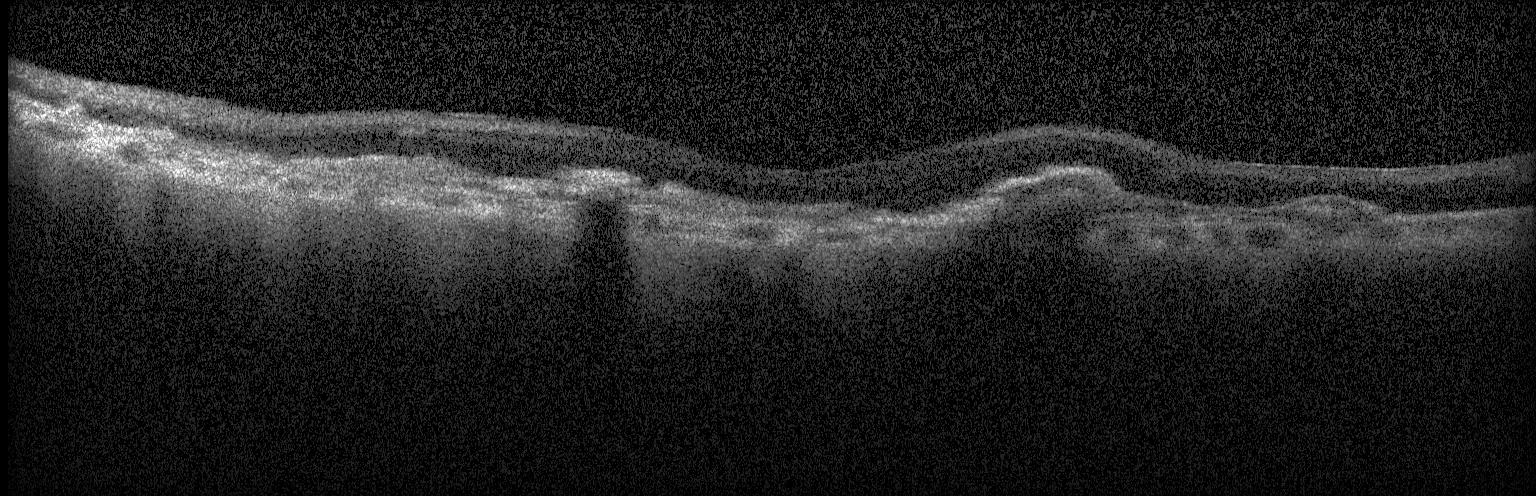
Spectral-domain OCT B-scan: a choroidal neovascular membrane.